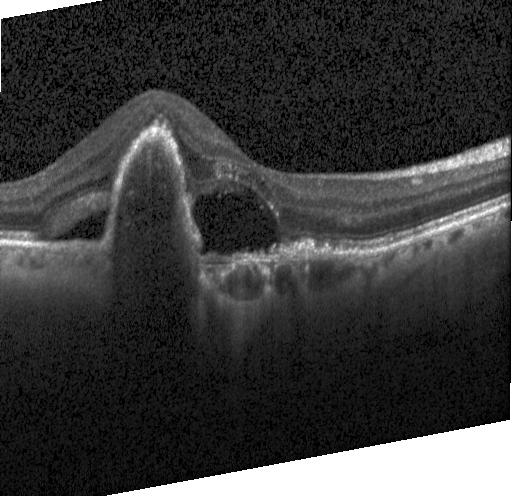 Impression: a choroidal neovascular membrane.